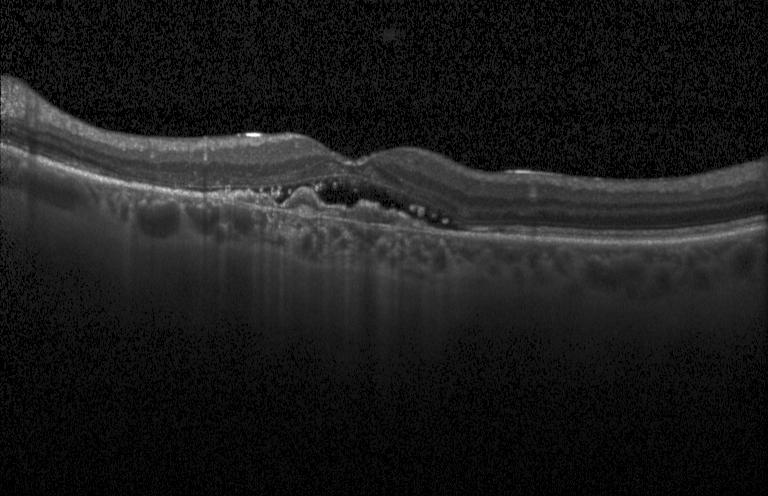

Optical coherence tomography B-scan.
Choroidal neovascularization.